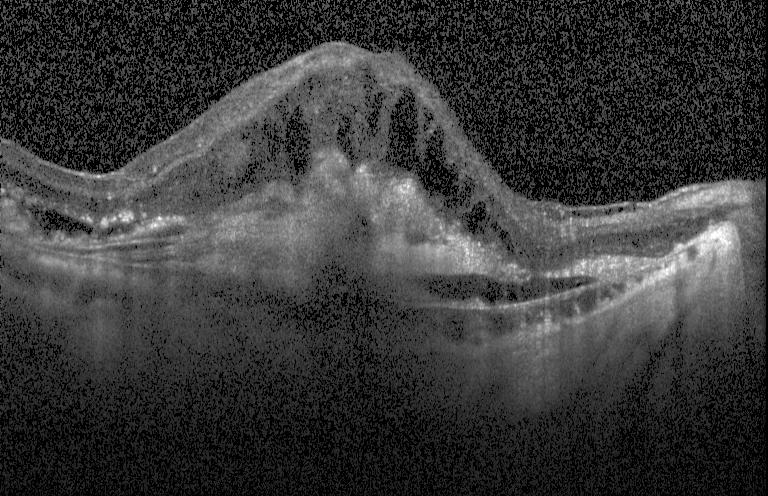
Spectral-domain OCT · horizontal scan through the fovea · optical coherence tomography B-scan.
Dx: choroidal neovascularization.